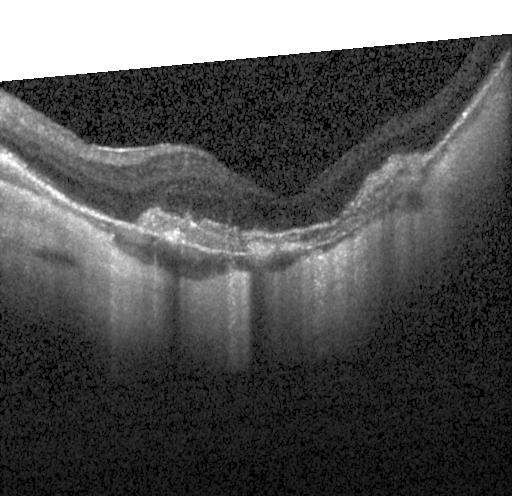

Retinal OCT B-scan
Choroidal neovascularization.